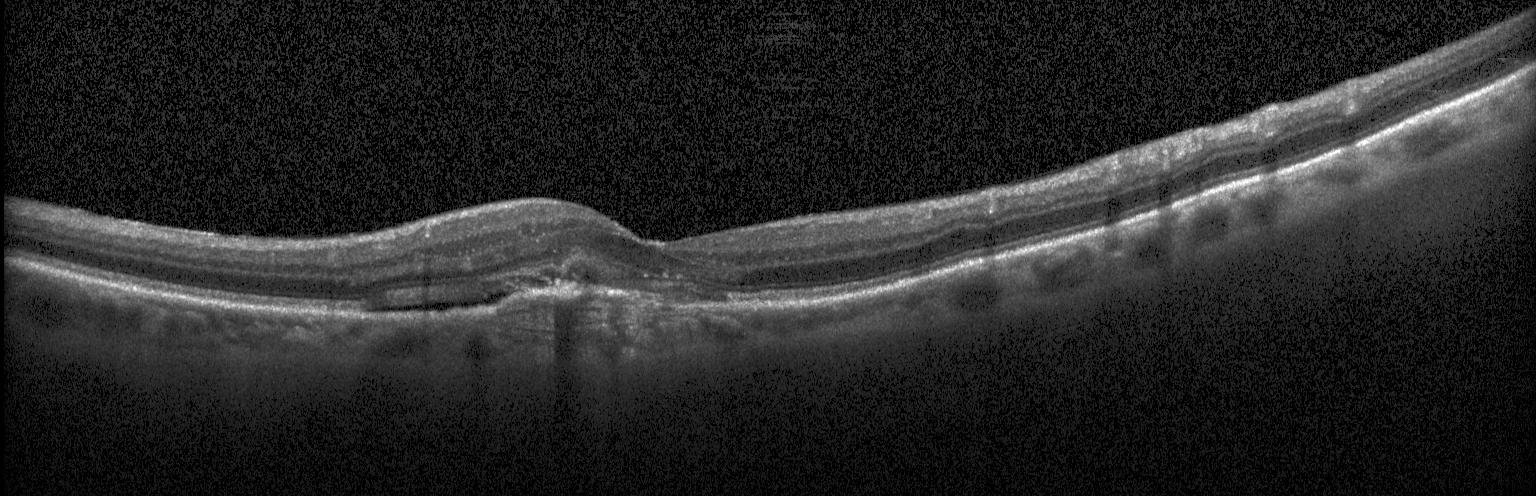 Dx: choroidal neovascularization.